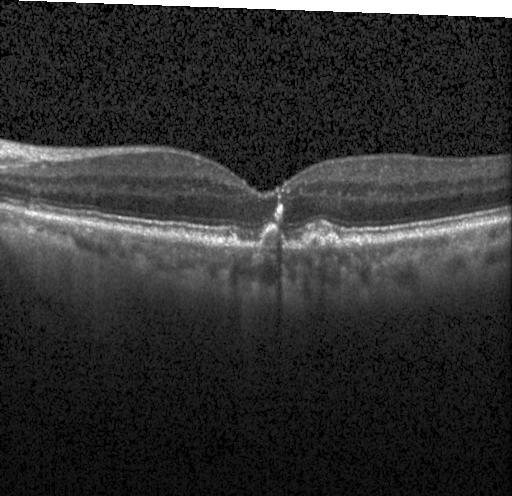
Optical coherence tomography B-scan. This B-scan demonstrates sub-RPE drusenoid deposits.